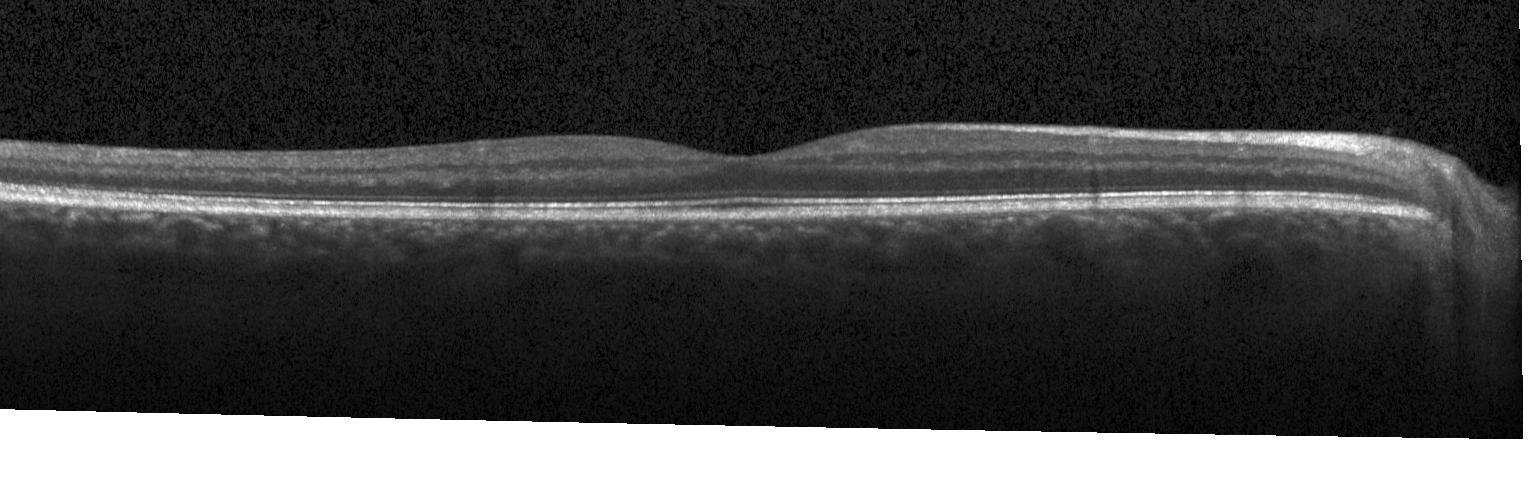 Optical coherence tomography scan — No choroidal neovascularization, diabetic macular edema, or drusen.